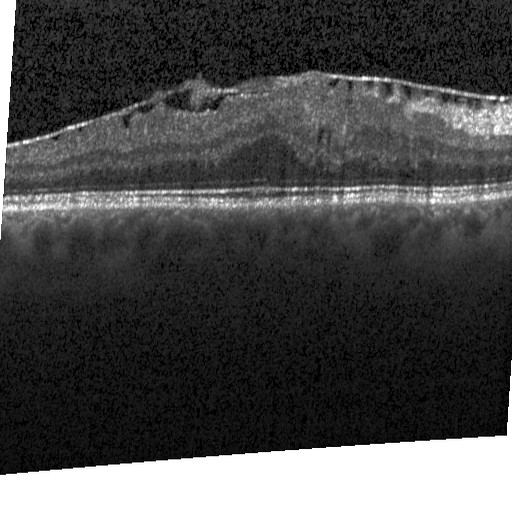
Diagnosis: diabetic macular edema.